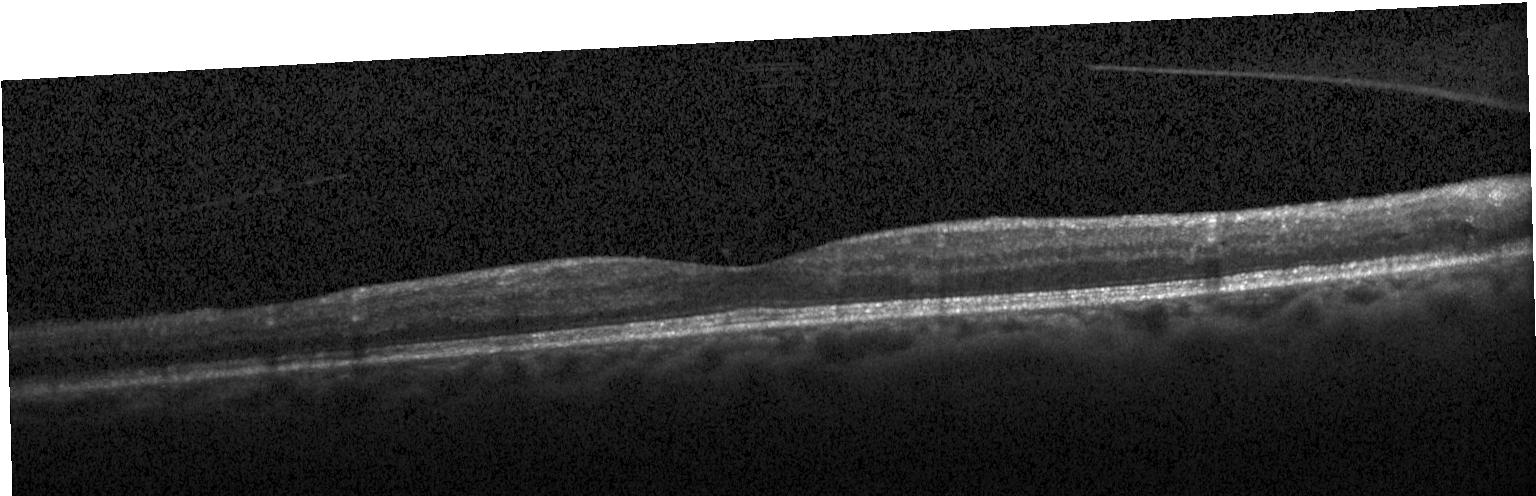

Finding: no evidence of choroidal neovascularization, diabetic macular edema, or drusen.